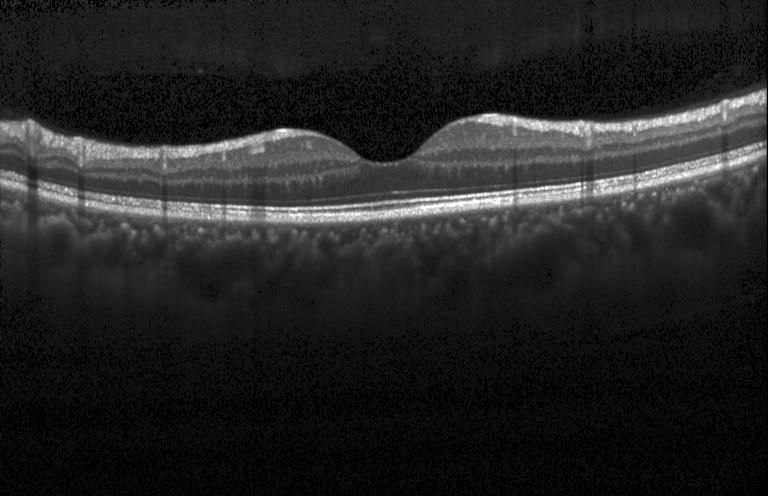 OCT line scan — Diagnosis: no choroidal neovascularization, diabetic macular edema, or drusen.